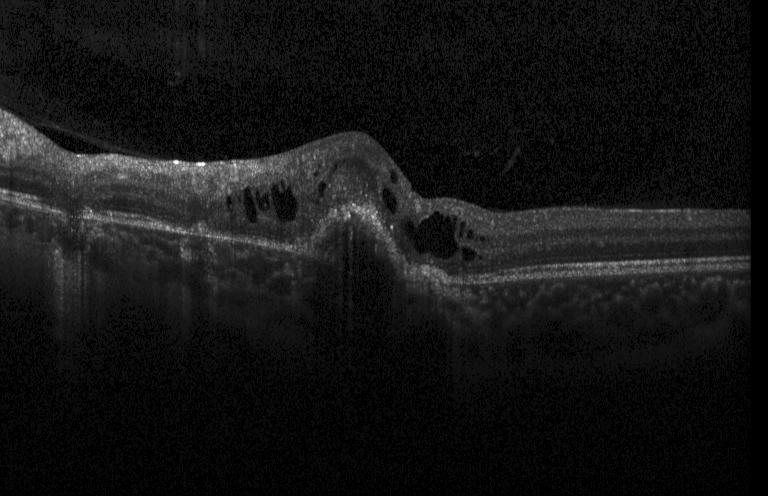 Finding: choroidal neovascularization.